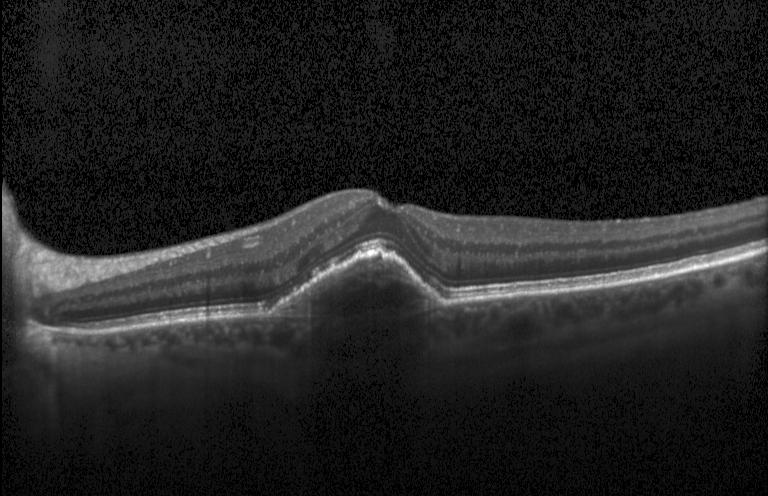

Spectral-domain optical coherence tomography. OCT B-scan — Impression: a choroidal neovascular membrane.